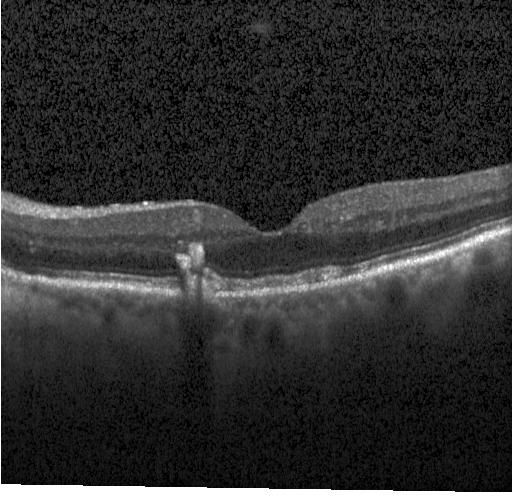
Spectral-domain OCT; optical coherence tomography B-scan.
Diagnosis: multiple drusen.